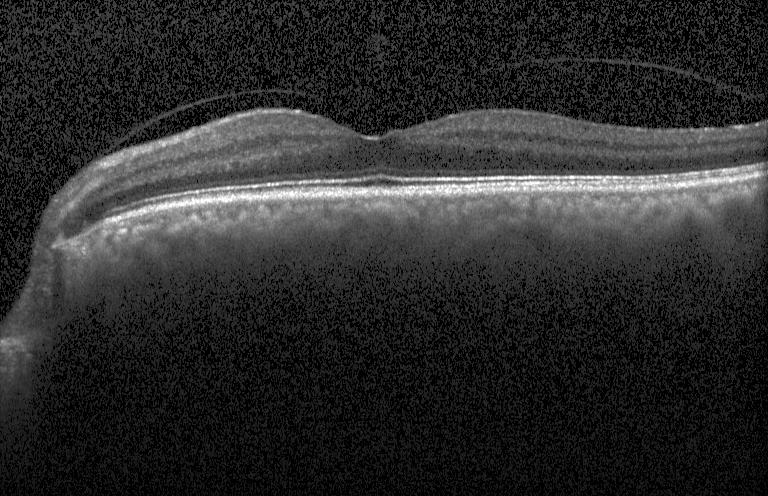
The scan shows no choroidal neovascularization, diabetic macular edema, or drusen.